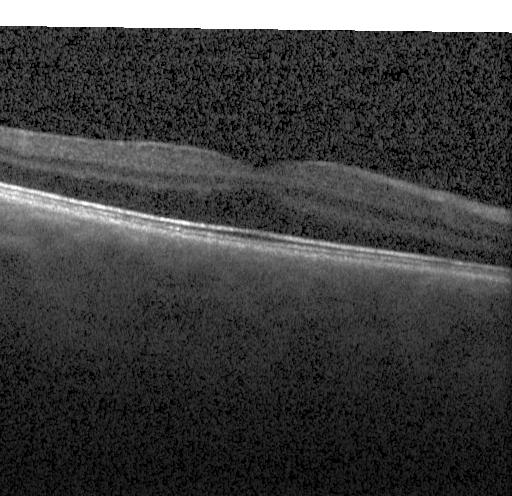

Spectral-domain OCT B-scan: no choroidal neovascularization, diabetic macular edema, or drusen.